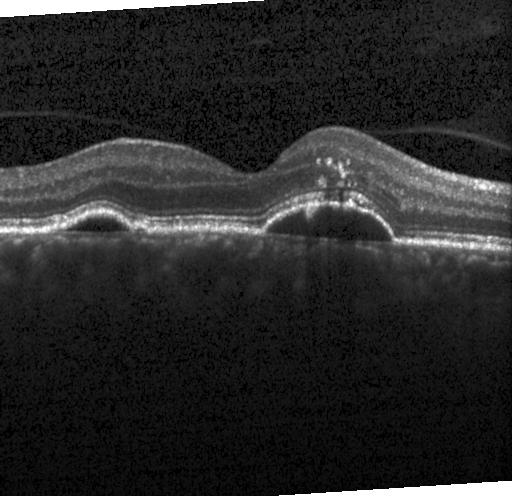 Instrument: Heidelberg Spectralis · spectral-domain optical coherence tomography · OCT line scan · horizontal scan through the fovea — Diagnosis: a choroidal neovascular membrane.